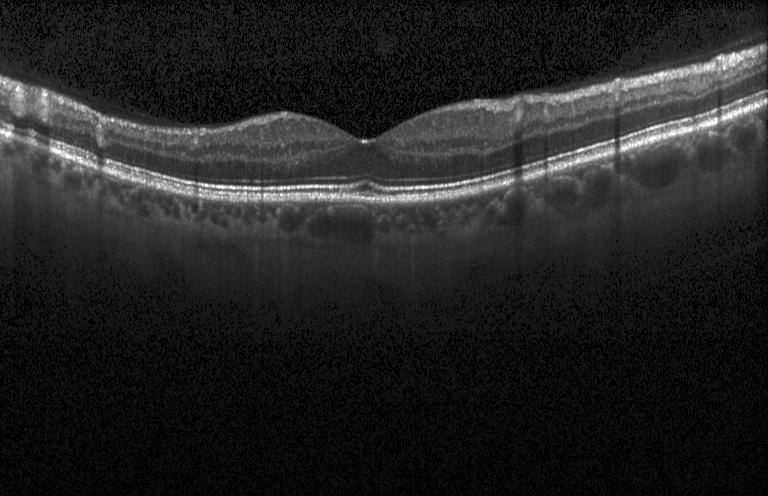 SD-OCT, instrument: Heidelberg Spectralis, OCT line scan, fovea-centered
Macular OCT: neither choroidal neovascularization, diabetic macular edema, nor drusen.